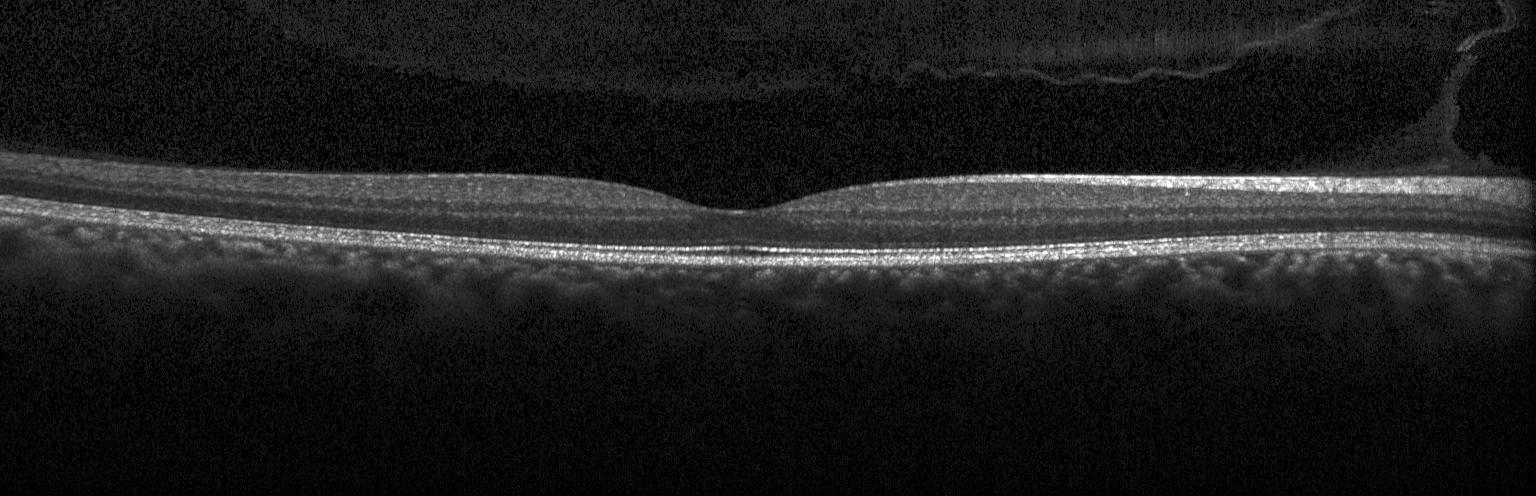
SD-OCT · optical coherence tomography scan · horizontal scan through the fovea · Heidelberg Spectralis — OCT finding: no choroidal neovascularization, diabetic macular edema, or drusen.